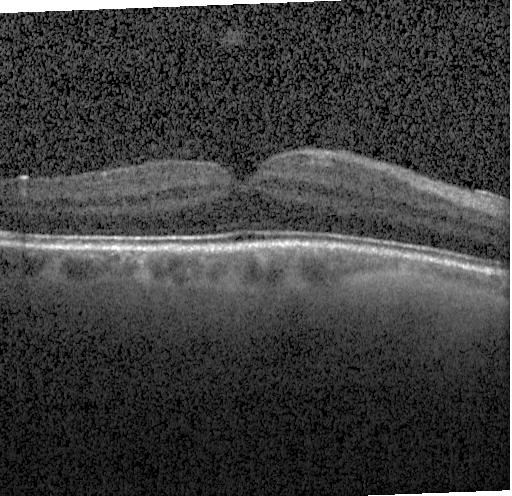

Assessment: no evidence of choroidal neovascularization, diabetic macular edema, or drusen.